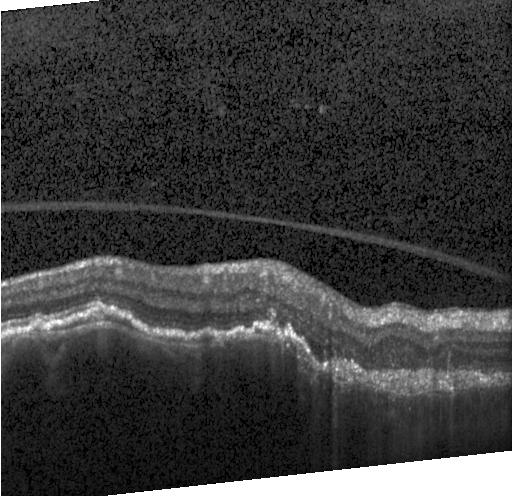
Fovea-centered, OCT line scan. This B-scan demonstrates a choroidal neovascular membrane.